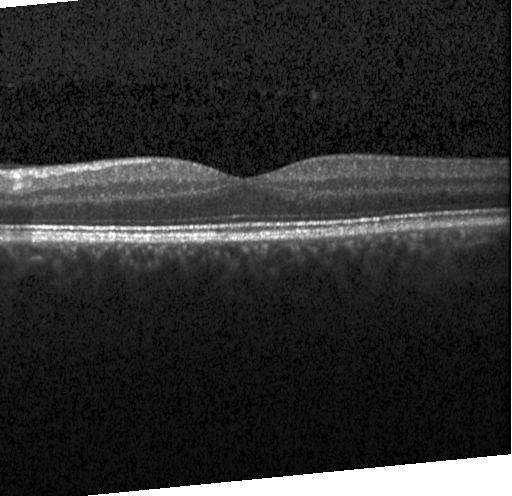

This B-scan demonstrates no choroidal neovascularization, no diabetic macular edema, and no drusen.